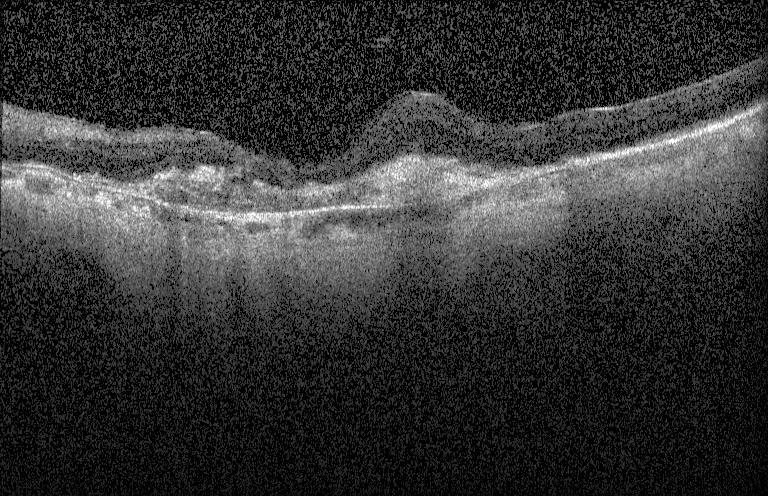 Fovea-centered; spectral-domain optical coherence tomography; retinal OCT B-scan
A choroidal neovascular membrane.